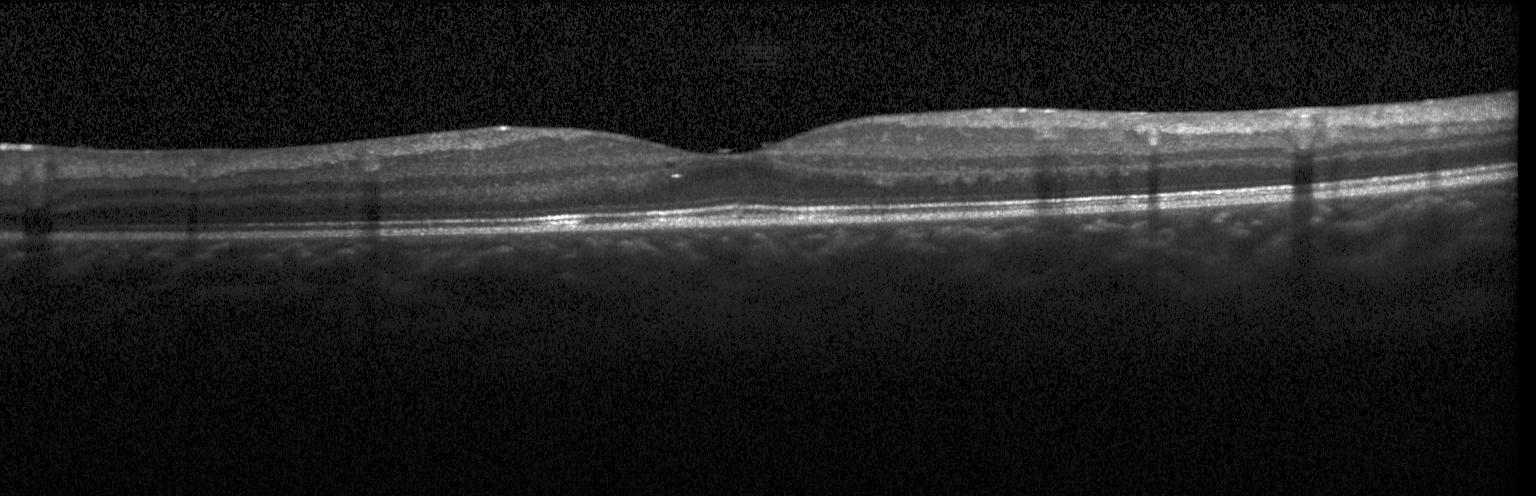
OCT finding: no evidence of choroidal neovascularization, diabetic macular edema, or drusen.